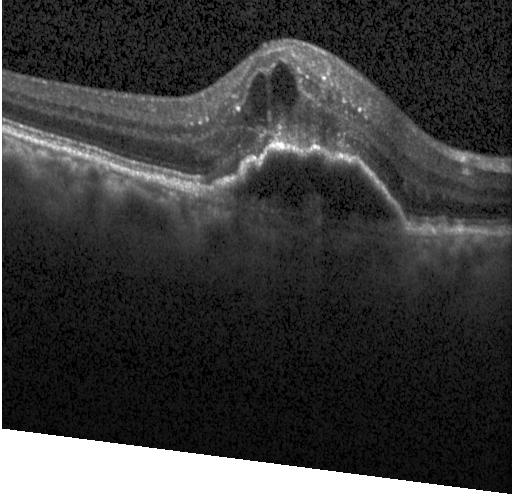

Impression: CNV.